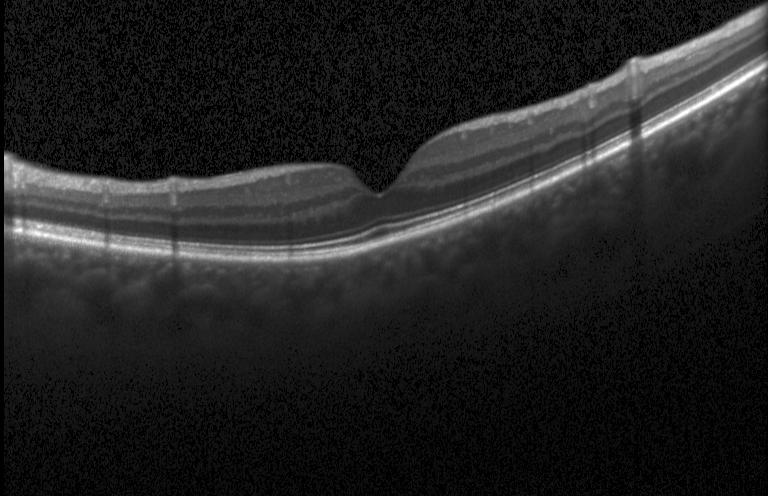

Retinal OCT B-scan
Finding: no choroidal neovascularization, diabetic macular edema, or drusen.